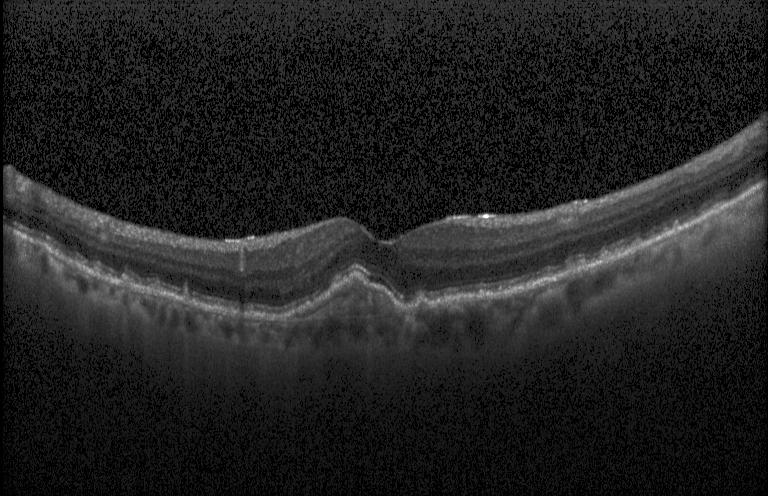
Centered on the fovea; optical coherence tomography B-scan; instrument: Heidelberg Spectralis; spectral-domain optical coherence tomography — Assessment: choroidal neovascularization.